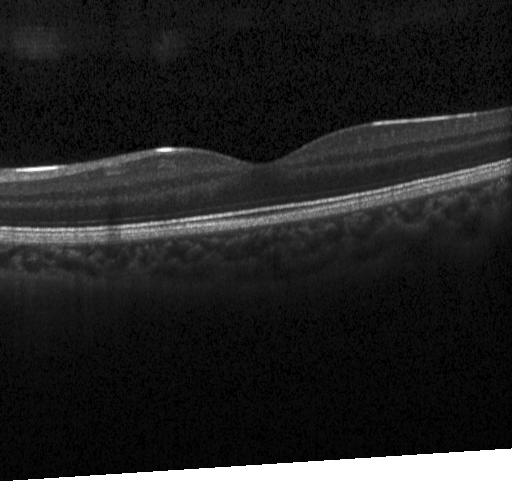
Retinal OCT cross-section.
Diagnosis: no CNV, no DME, and no drusen.